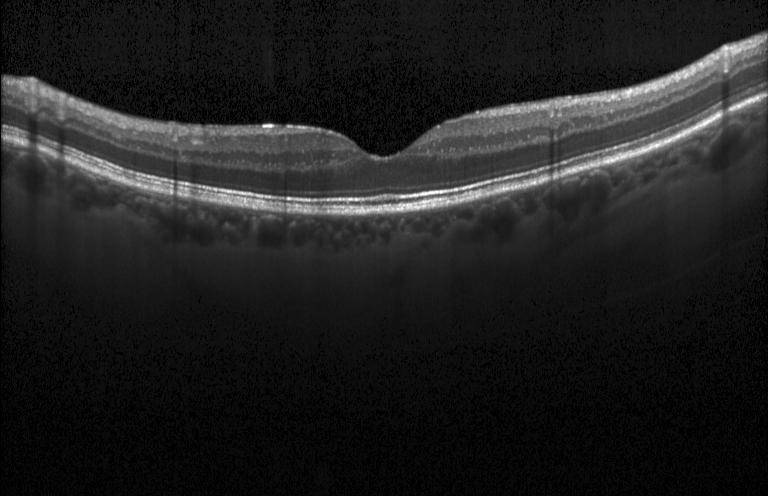 Impression: no evidence of CNV, DME, or drusen.